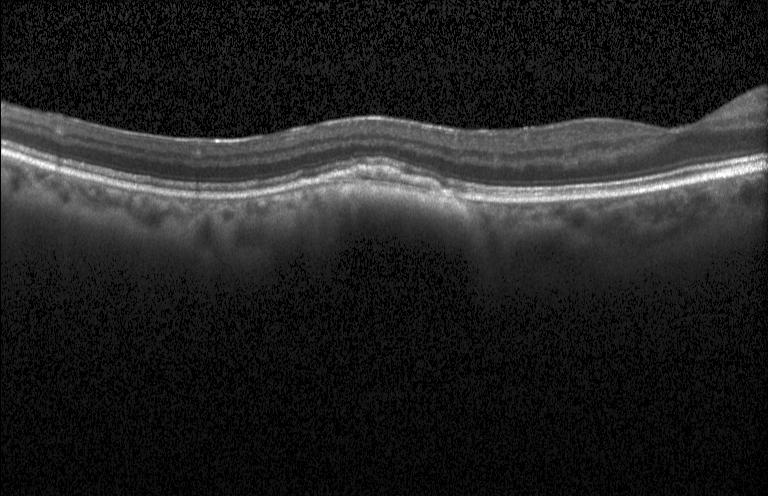
Instrument: Heidelberg Spectralis · optical coherence tomography scan · spectral-domain optical coherence tomography · fovea-centered
Finding: a choroidal neovascular membrane.